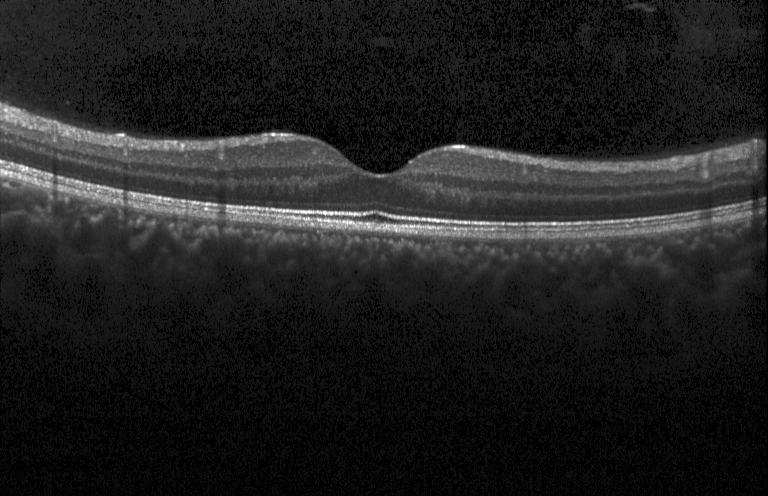
OCT B-scan showing neither choroidal neovascularization, diabetic macular edema, nor drusen.